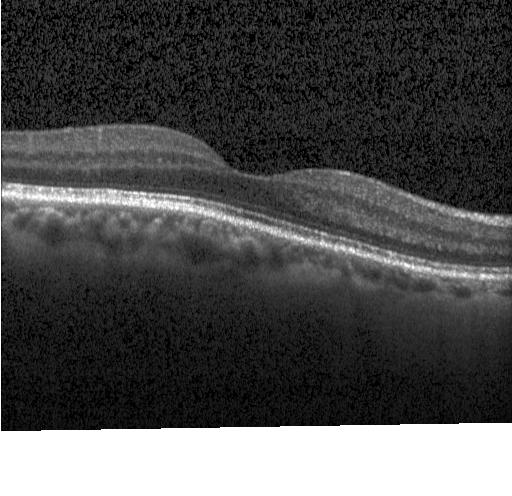 Spectral-domain optical coherence tomography; acquired on a Heidelberg Spectralis; OCT line scan
Macular OCT: no choroidal neovascularization, no diabetic macular edema, and no drusen.